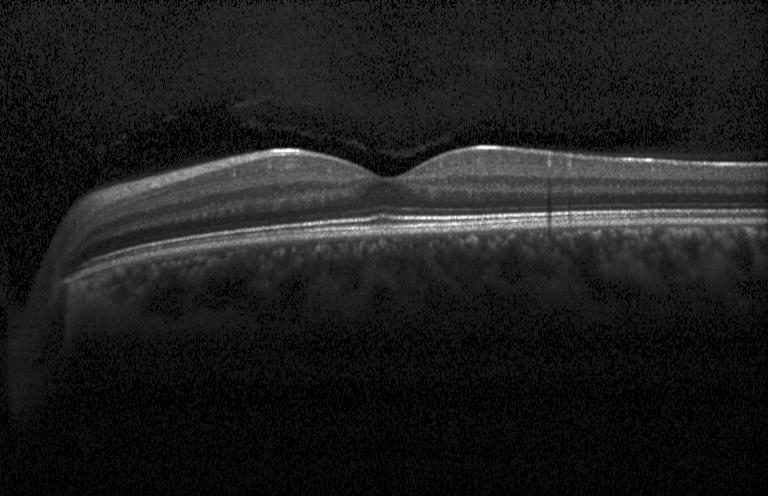 Heidelberg Spectralis OCT system; SD-OCT; retinal OCT B-scan
The scan shows no choroidal neovascularization, diabetic macular edema, or drusen.